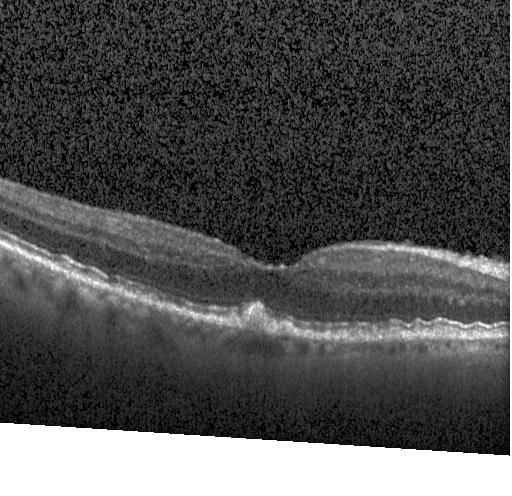

Fovea-centered. SD-OCT. Optical coherence tomography B-scan. Heidelberg Spectralis — This B-scan demonstrates multiple drusen.